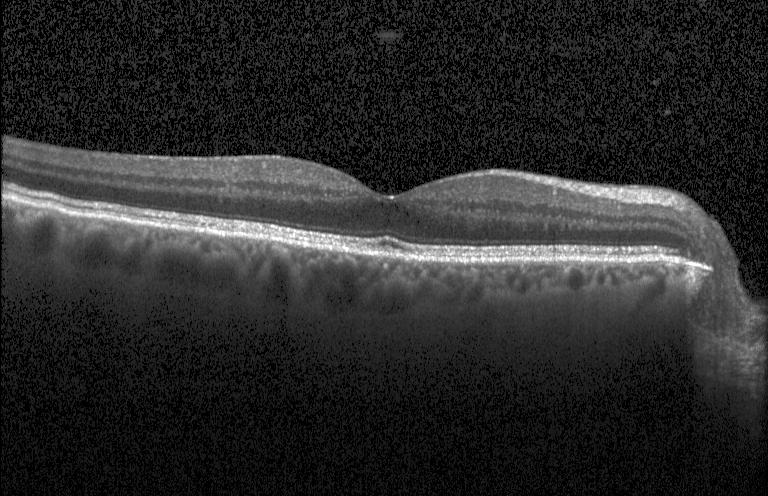
Fovea-centered, SD-OCT, OCT line scan, acquired on a Heidelberg Spectralis — Macular OCT: no choroidal neovascularization, diabetic macular edema, or drusen.